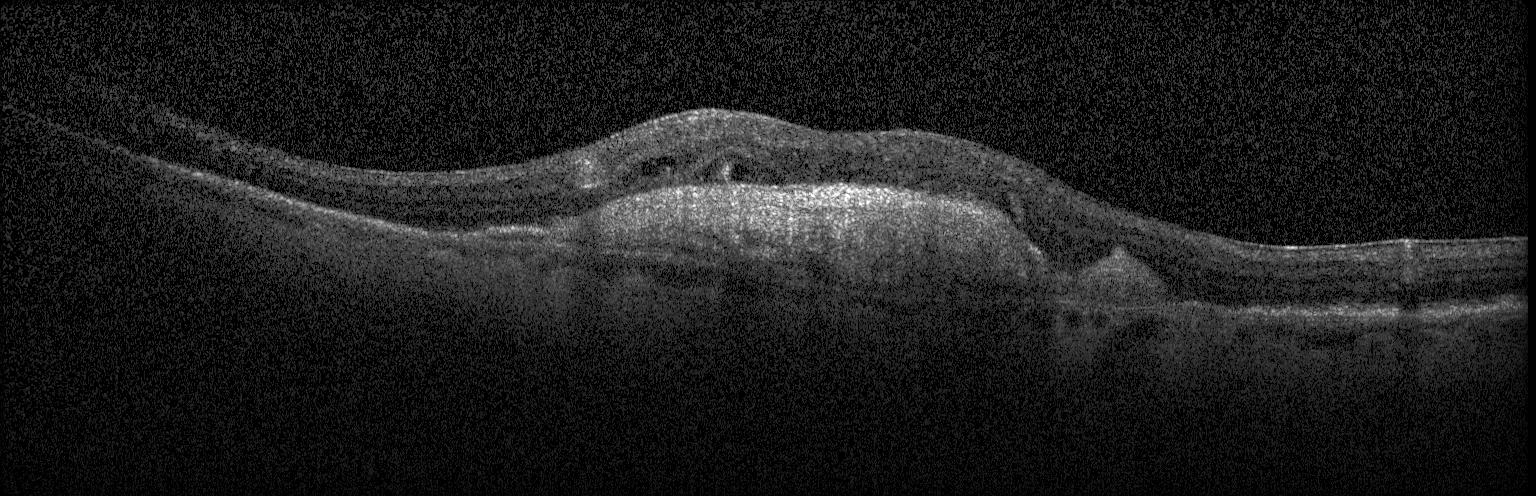
Spectral-domain optical coherence tomography · acquired on a Heidelberg Spectralis · through the macula · retinal OCT B-scan
Dx: choroidal neovascularization (CNV).